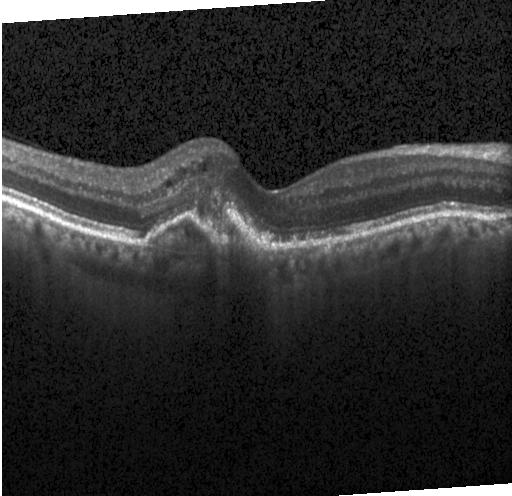

Retinal OCT B-scan, SD-OCT.
Diagnosis: a choroidal neovascular membrane.